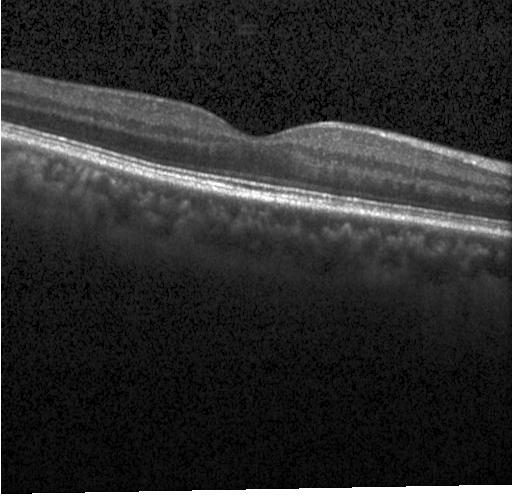

Heidelberg Spectralis OCT system · OCT B-scan · spectral-domain OCT
Finding: no CNV, no DME, and no drusen.